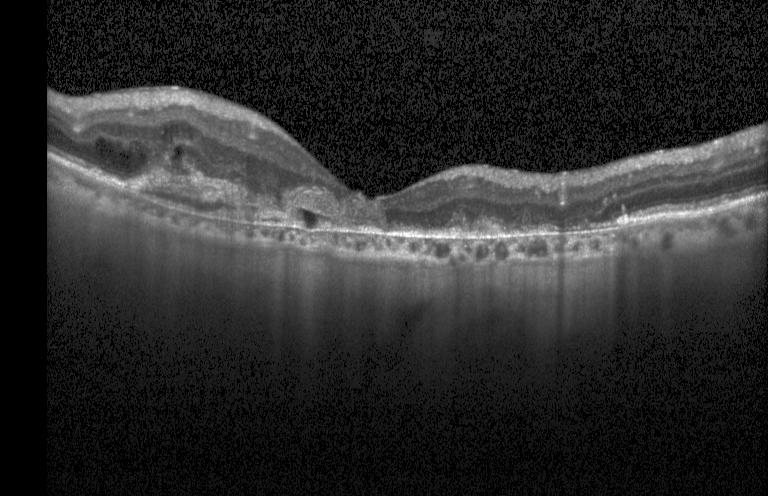 Optical coherence tomography B-scan
Diagnosis: CNV.